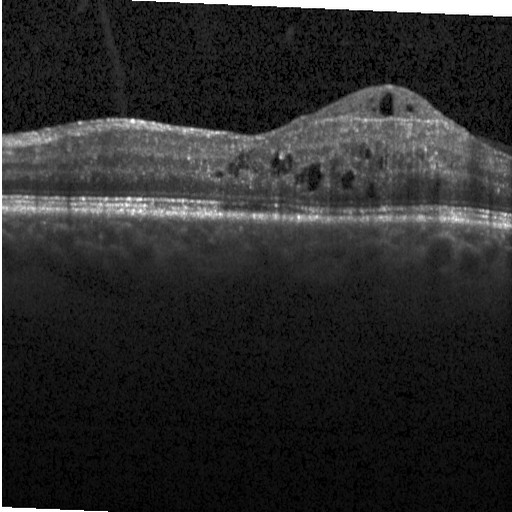 Heidelberg Spectralis. Retinal OCT B-scan.
The scan shows diabetic macular edema.